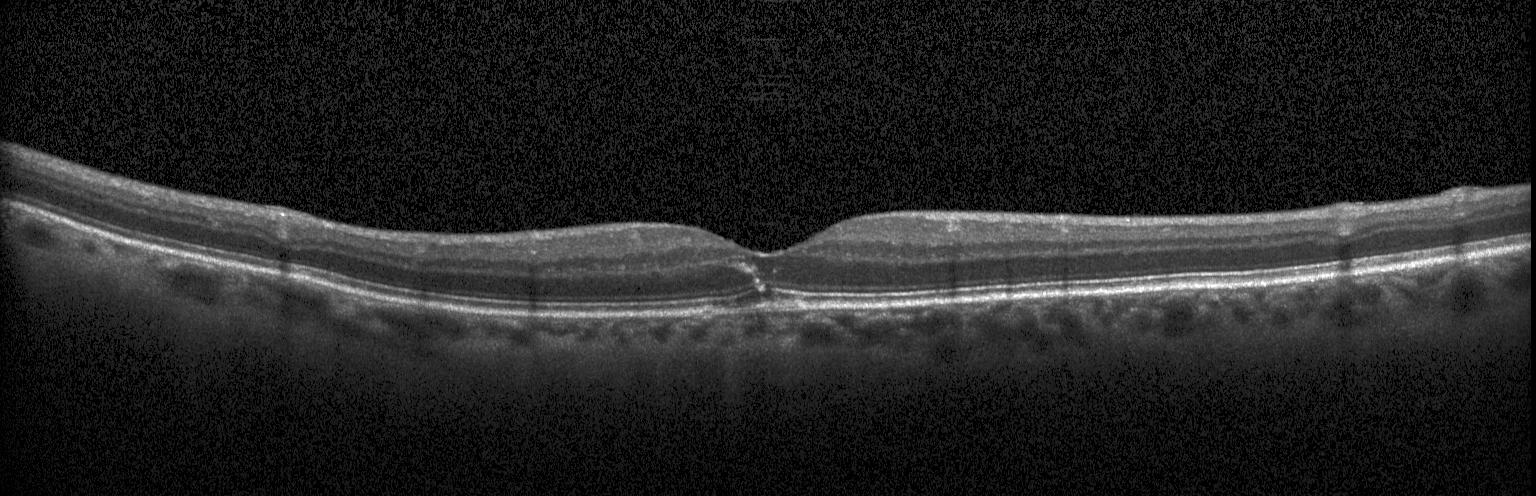

Spectral-domain optical coherence tomography, instrument: Heidelberg Spectralis, horizontal scan through the fovea, OCT B-scan.
Macular OCT: a choroidal neovascular membrane.